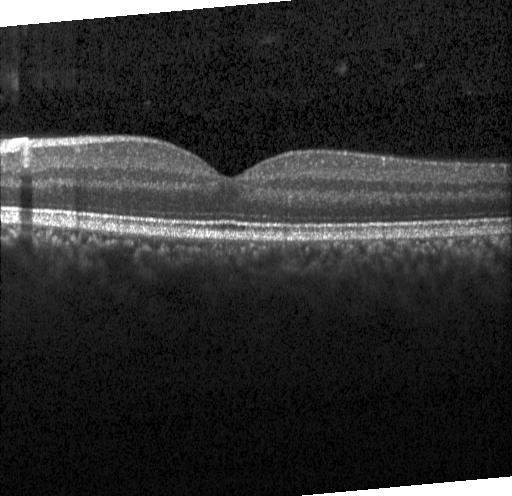 The scan shows neither choroidal neovascularization, diabetic macular edema, nor drusen.